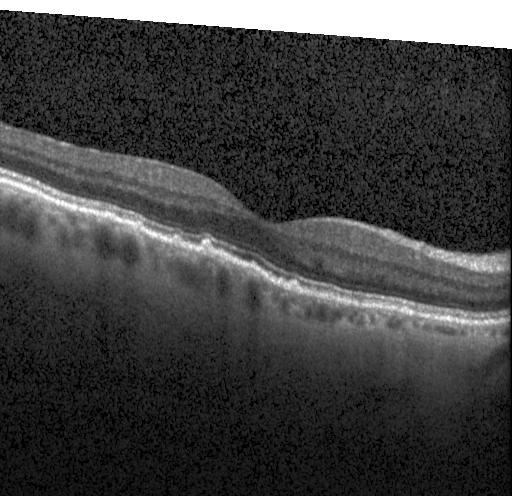 SD-OCT; OCT B-scan.
Sub-RPE drusenoid deposits.